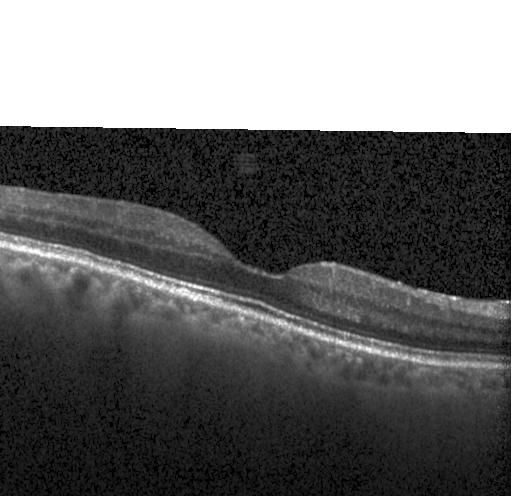
Retinal OCT cross-section; spectral-domain optical coherence tomography. Diagnosis: no evidence of choroidal neovascularization, diabetic macular edema, or drusen.